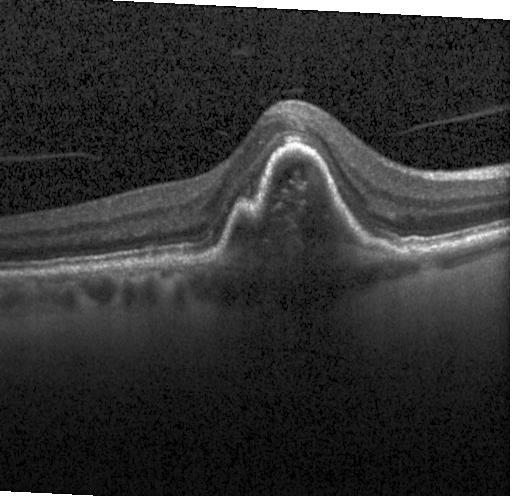 Macular OCT: a choroidal neovascular membrane.